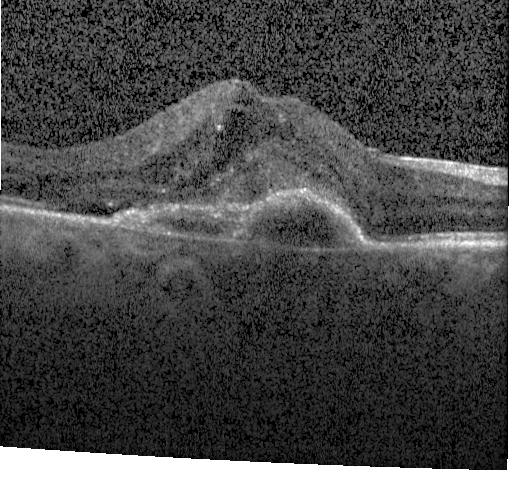
OCT line scan — Diagnosis: choroidal neovascularization.